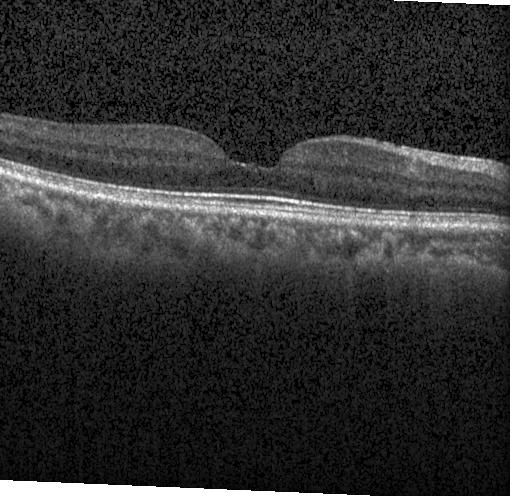
Optical coherence tomography scan. Spectral-domain OCT — The scan shows no CNV, no DME, and no drusen.